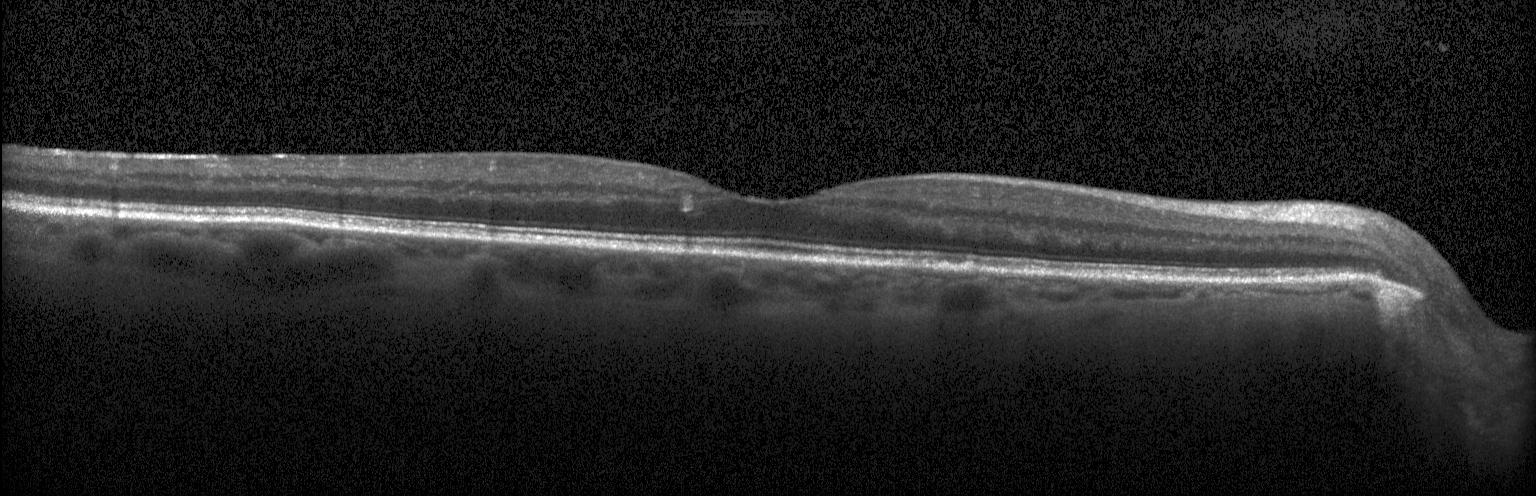
Optical coherence tomography scan
Impression: no evidence of CNV, DME, or drusen.